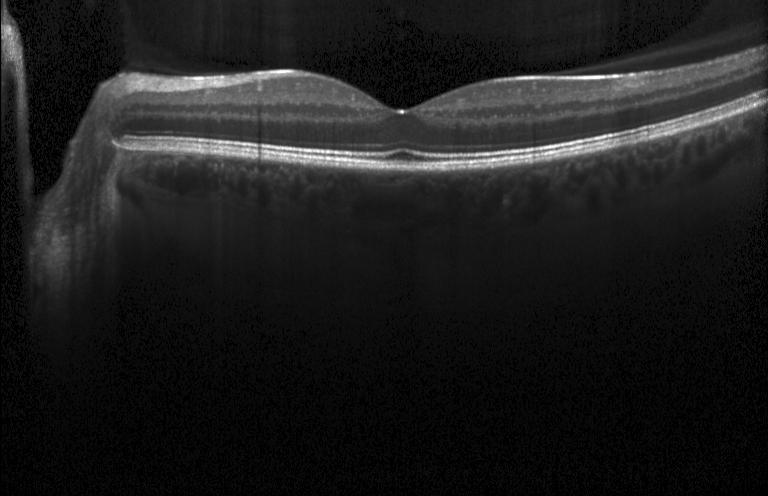

Optical coherence tomography B-scan, spectral-domain optical coherence tomography
Impression: no choroidal neovascularization, no diabetic macular edema, and no drusen.